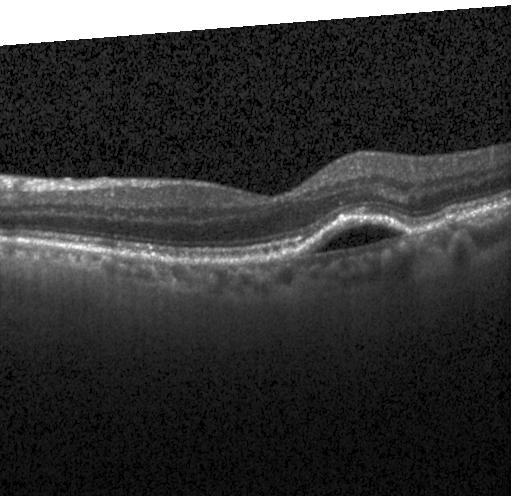 Retinal OCT B-scan; spectral-domain optical coherence tomography; horizontal scan through the fovea; instrument: Heidelberg Spectralis.
Impression: choroidal neovascularization.